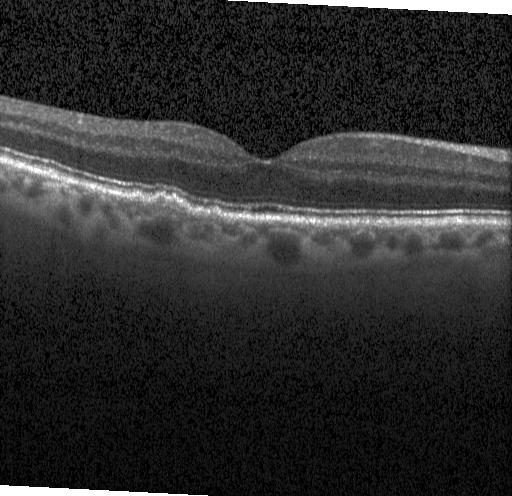 OCT B-scan, centered on the fovea.
Drusen.